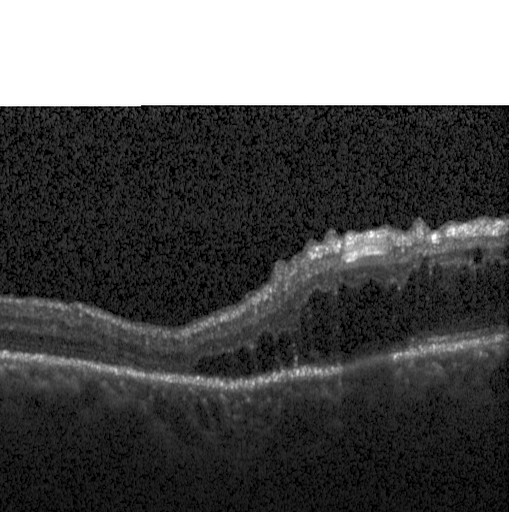

Macular OCT demonstrating diabetic macular edema (DME).